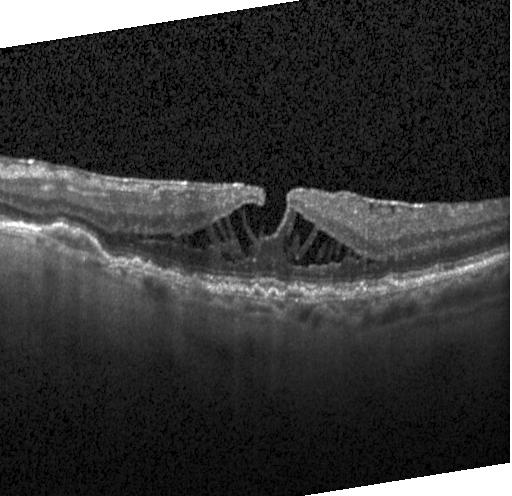
OCT finding: diabetic macular edema.